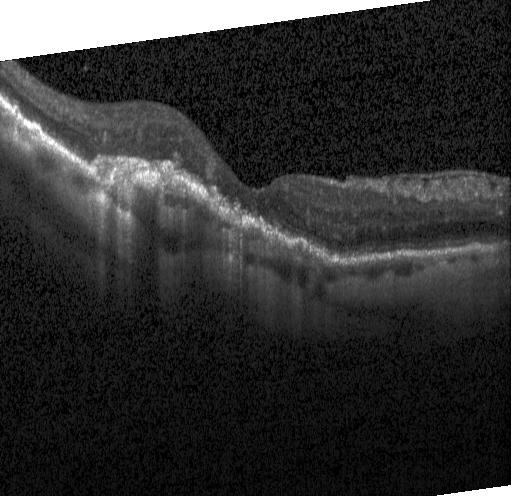

Finding: a choroidal neovascular membrane.